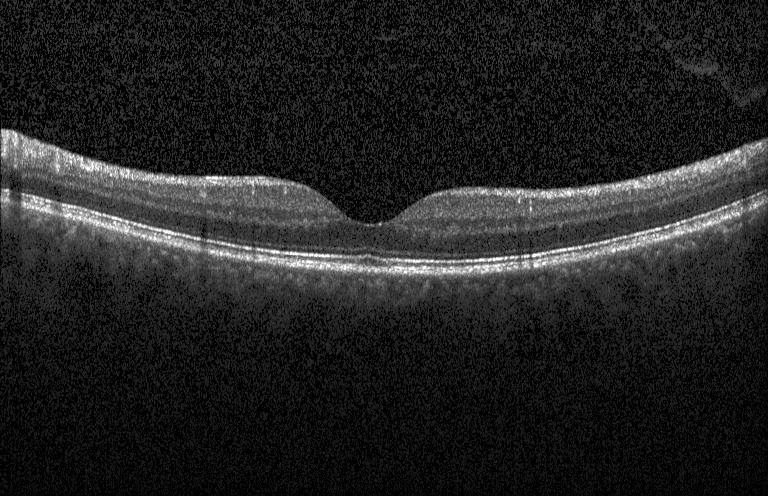 Spectral-domain OCT B-scan: no choroidal neovascularization, diabetic macular edema, or drusen.